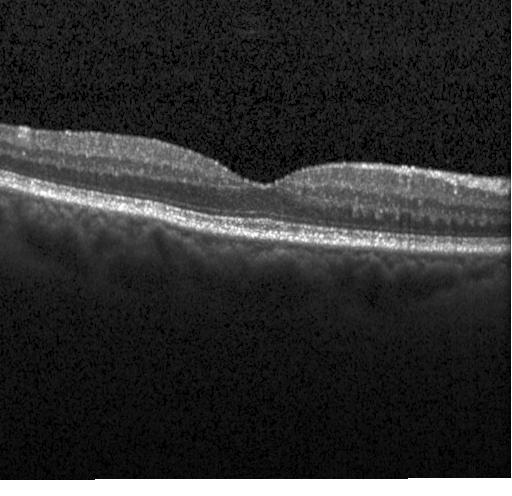

Spectral-domain optical coherence tomography · OCT B-scan · Heidelberg Spectralis · fovea-centered — Impression: no choroidal neovascularization, no diabetic macular edema, and no drusen.